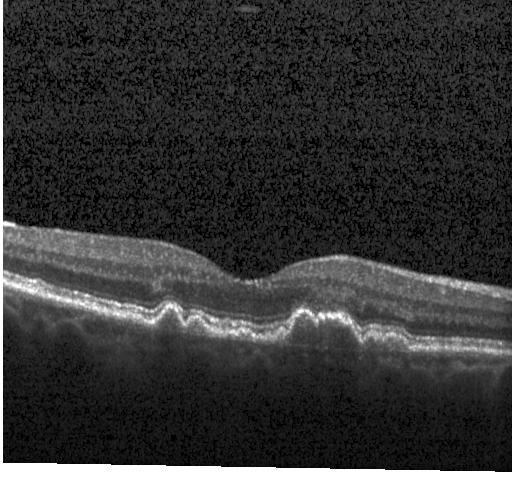 Optical coherence tomography B-scan, acquired on a Heidelberg Spectralis.
The scan shows sub-RPE drusenoid deposits.